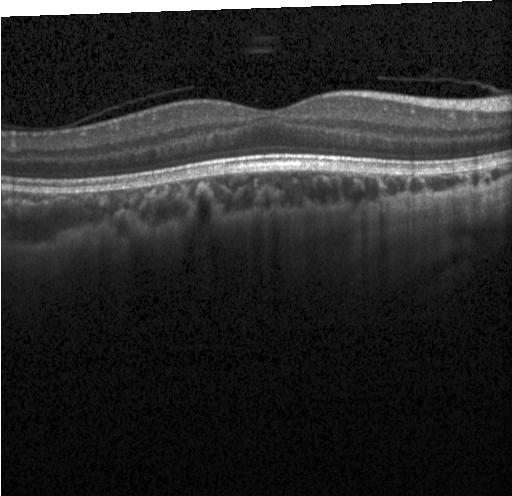
Spectral-domain OCT; centered on the fovea; retinal OCT B-scan. Diagnosis: neither choroidal neovascularization, diabetic macular edema, nor drusen.